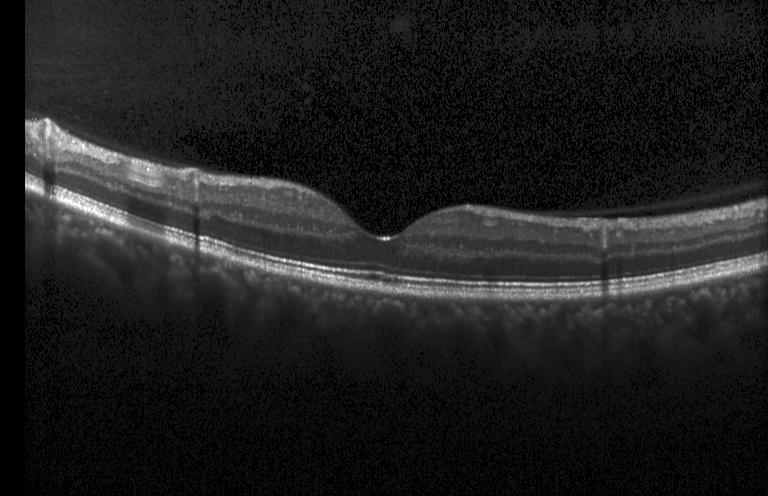 Dx: no choroidal neovascularization, diabetic macular edema, or drusen.